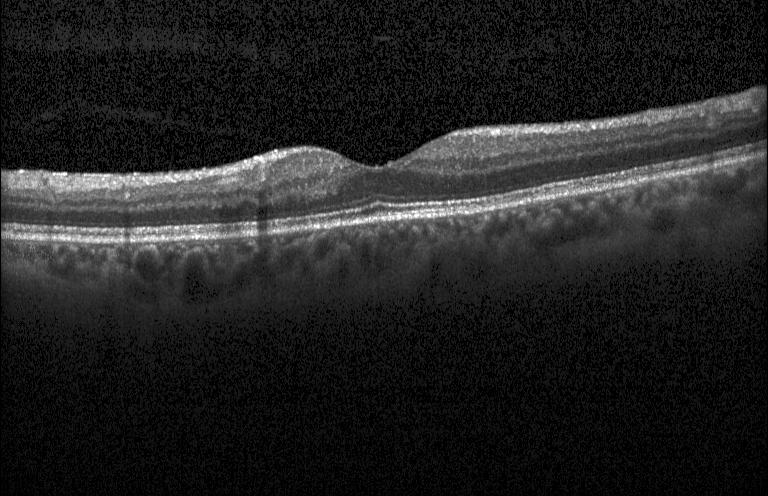
Acquired on a Heidelberg Spectralis, optical coherence tomography scan.
Impression: neither choroidal neovascularization, diabetic macular edema, nor drusen.